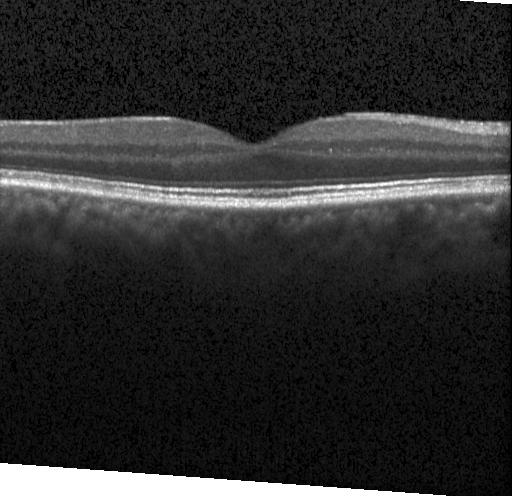 Finding: no evidence of choroidal neovascularization, diabetic macular edema, or drusen.